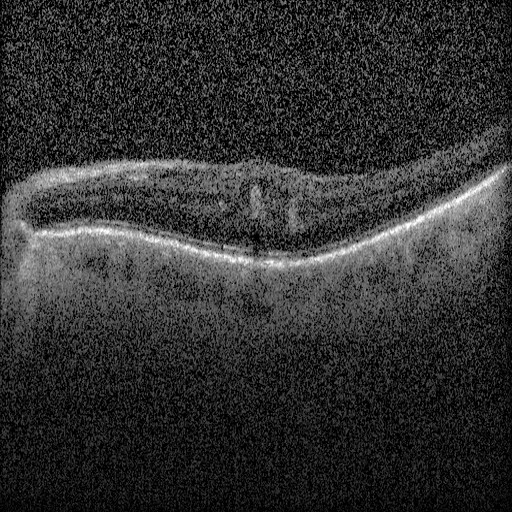

Spectral-domain OCT B-scan: diabetic macular edema.